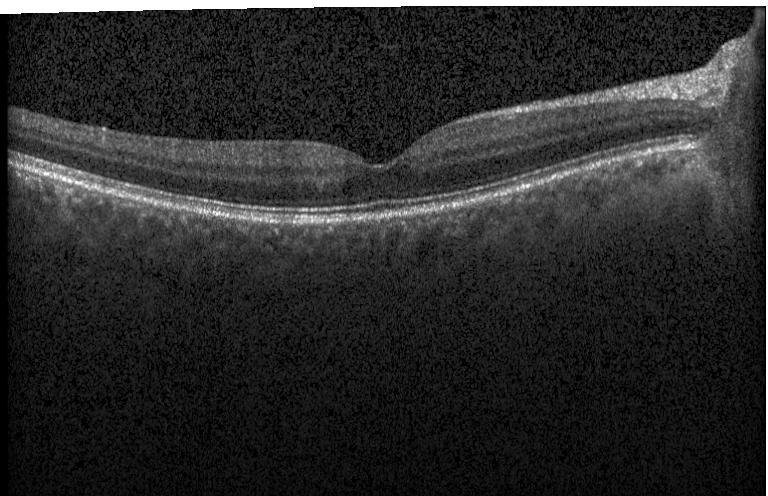

OCT B-scan
OCT finding: no evidence of CNV, DME, or drusen.